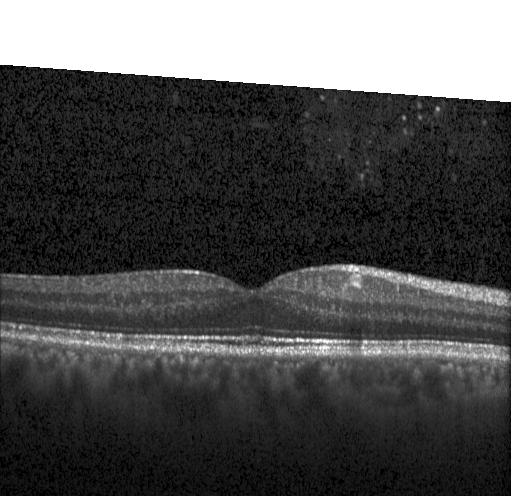
OCT line scan — Impression: no evidence of CNV, DME, or drusen.